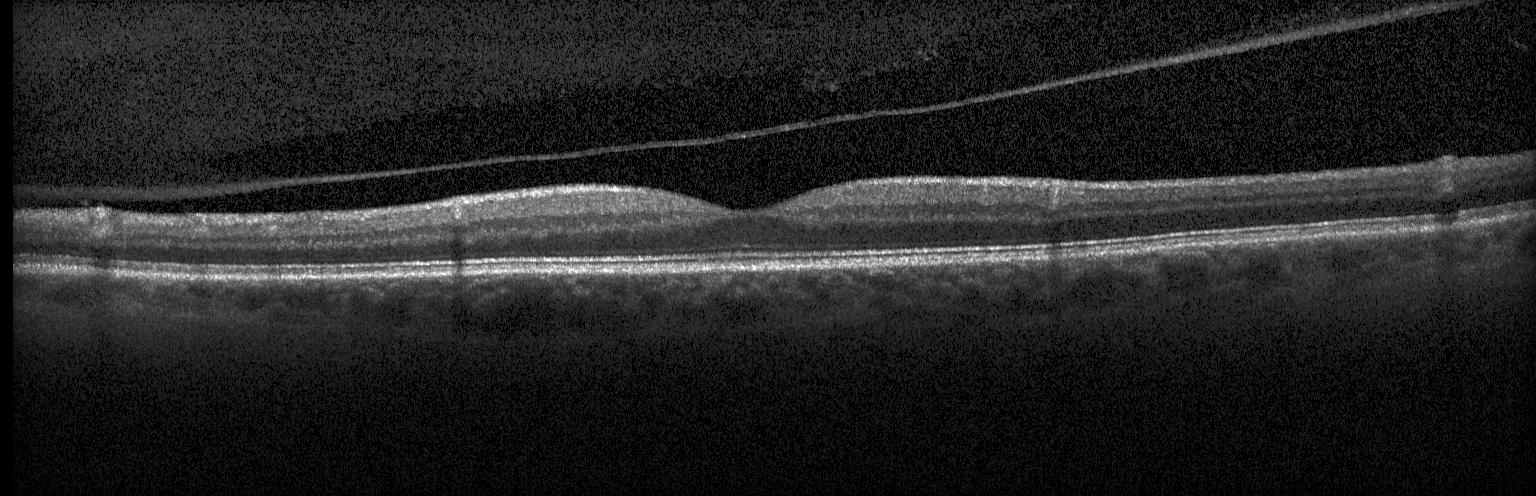 Retinal OCT cross-section showing no CNV, no DME, and no drusen.